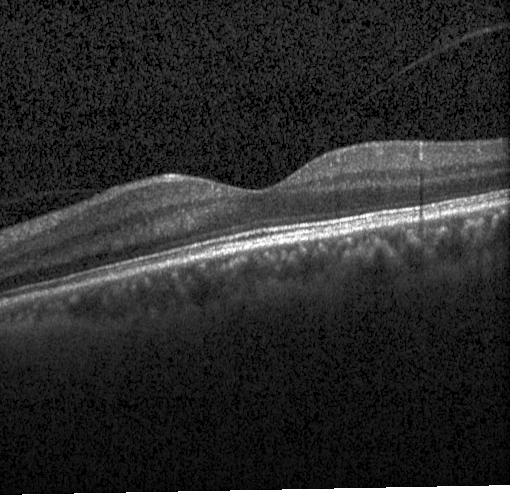

OCT scan showing no choroidal neovascularization, no diabetic macular edema, and no drusen.